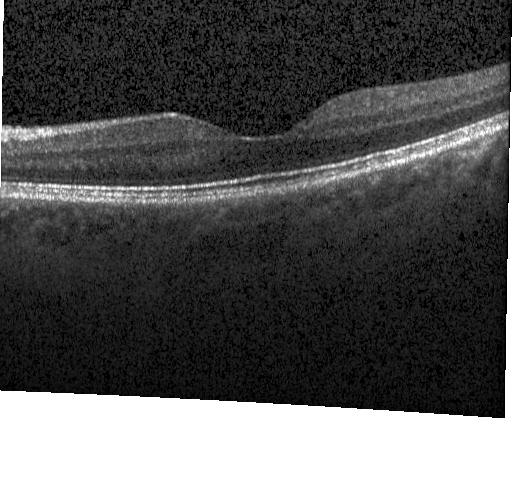

Macular OCT: no choroidal neovascularization, no diabetic macular edema, and no drusen.